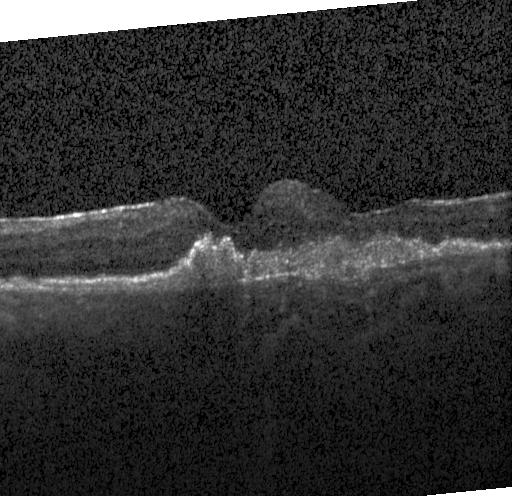
OCT line scan. Through the macula — This B-scan demonstrates choroidal neovascularization.